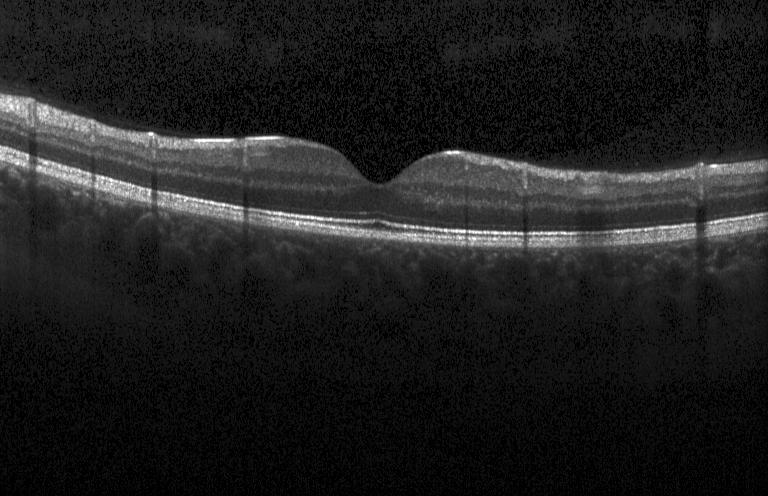 Finding: no evidence of choroidal neovascularization, diabetic macular edema, or drusen.